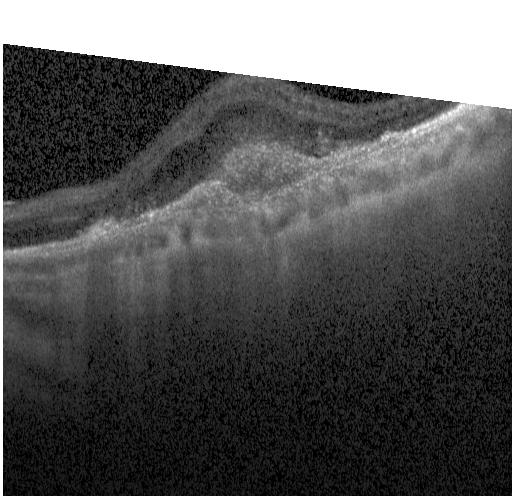

Macular OCT: a choroidal neovascular membrane.